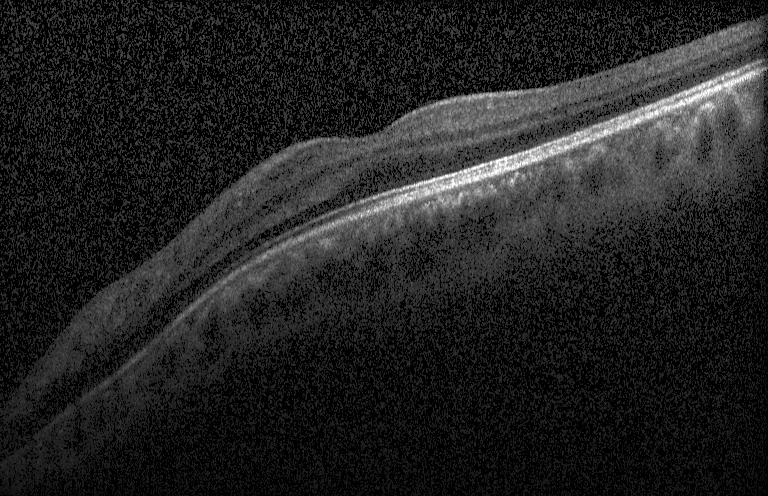
Diagnosis: no choroidal neovascularization, no diabetic macular edema, and no drusen.